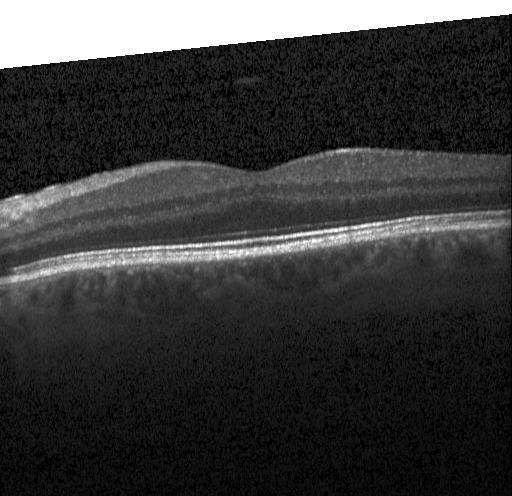

OCT line scan — Macular OCT: no choroidal neovascularization, no diabetic macular edema, and no drusen.